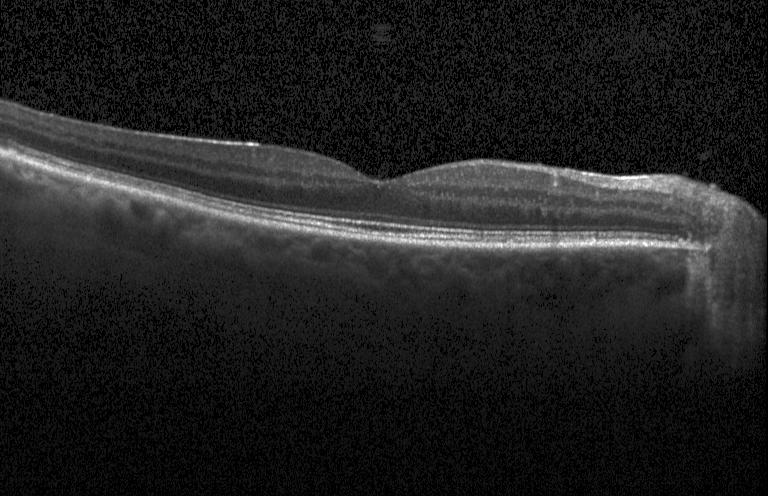 OCT B-scan showing no evidence of choroidal neovascularization, diabetic macular edema, or drusen.